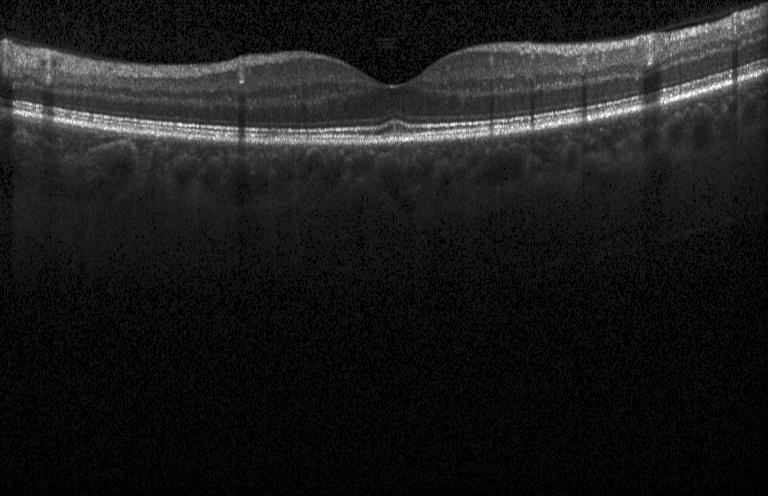 Instrument: Heidelberg Spectralis, optical coherence tomography B-scan, spectral-domain optical coherence tomography.
Dx: neither CNV, DME, nor drusen.